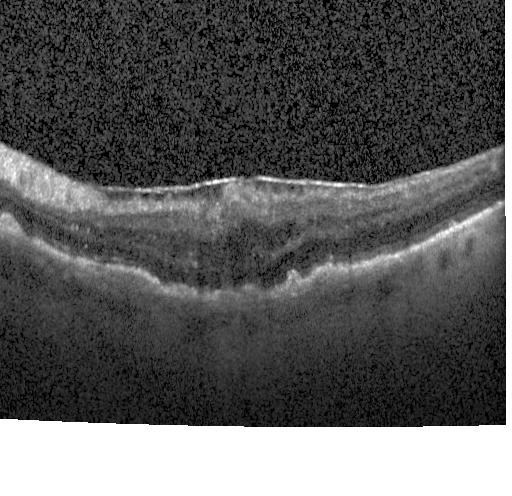 Finding: a choroidal neovascular membrane.